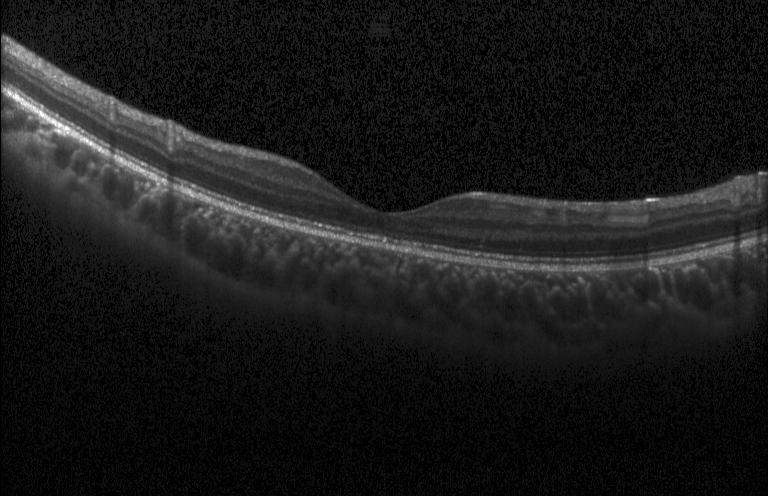

Assessment: no choroidal neovascularization, no diabetic macular edema, and no drusen.